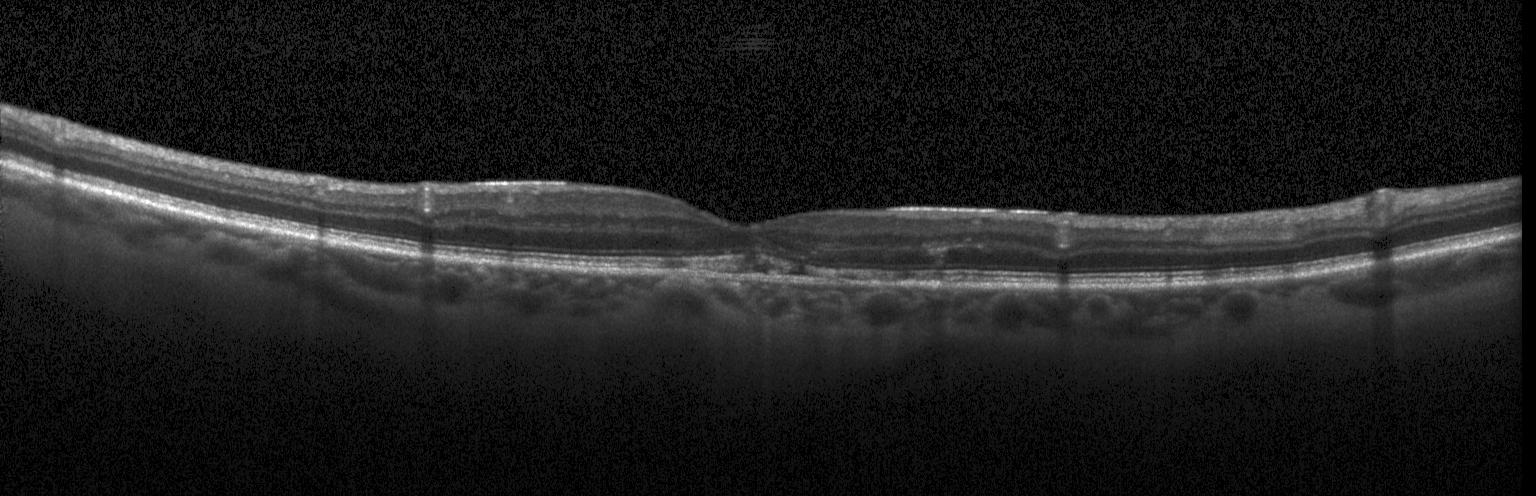
Impression: choroidal neovascularization (CNV).